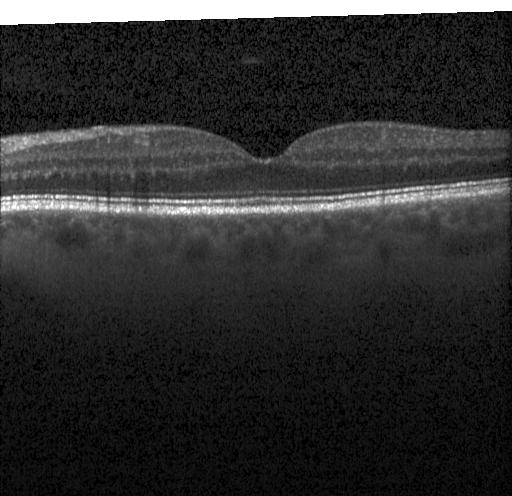

Impression: no choroidal neovascularization, diabetic macular edema, or drusen.